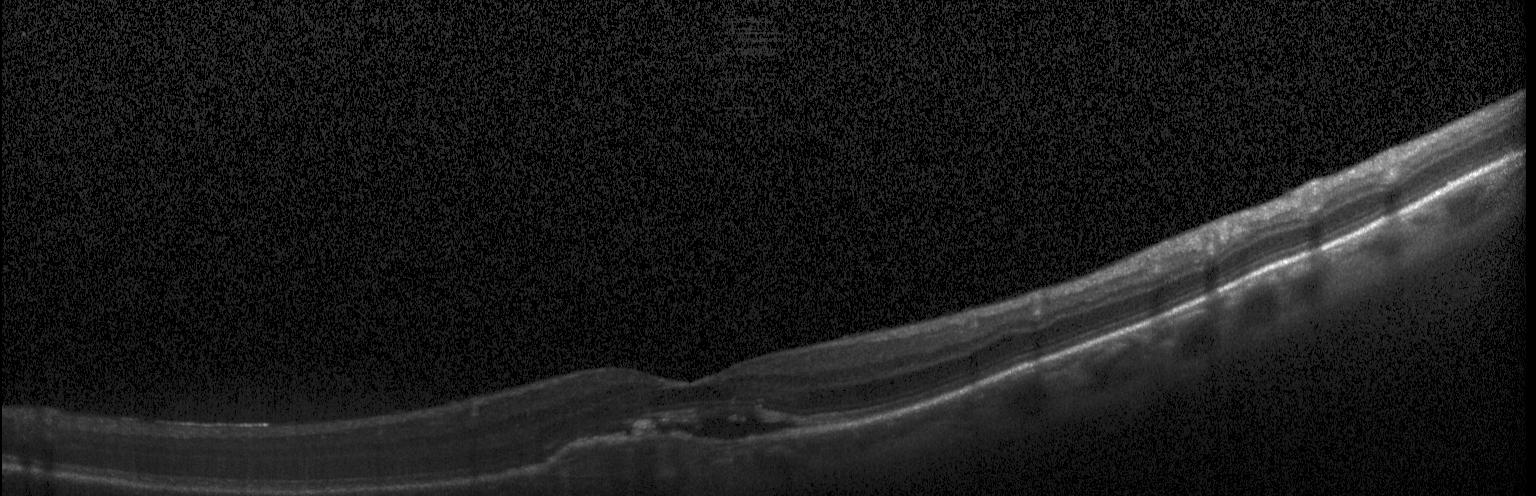
Macular OCT: choroidal neovascularization.